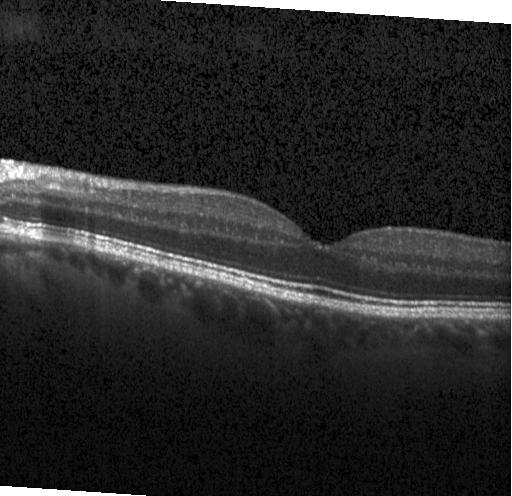

Spectral-domain optical coherence tomography, optical coherence tomography scan, acquired on a Heidelberg Spectralis, centered on the fovea.
Assessment: no choroidal neovascularization, no diabetic macular edema, and no drusen.